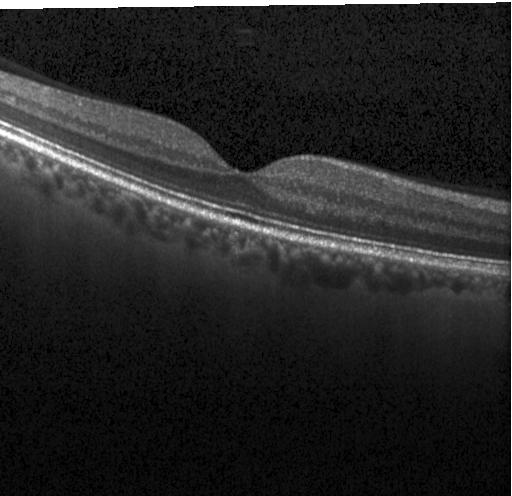
Retinal OCT cross-section — Impression: neither choroidal neovascularization, diabetic macular edema, nor drusen.